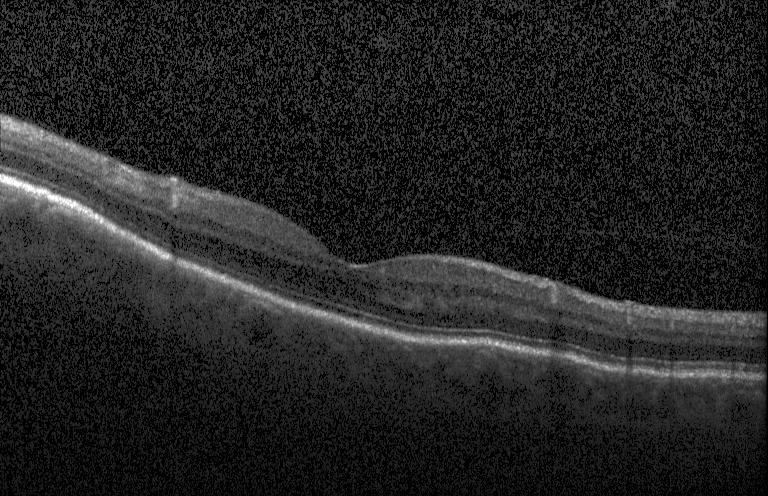
Diagnosis: no CNV, DME, or drusen.